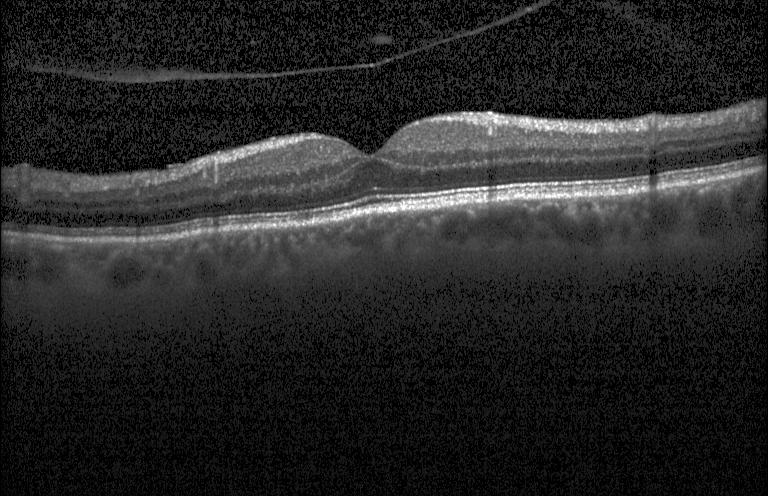
No evidence of CNV, DME, or drusen.